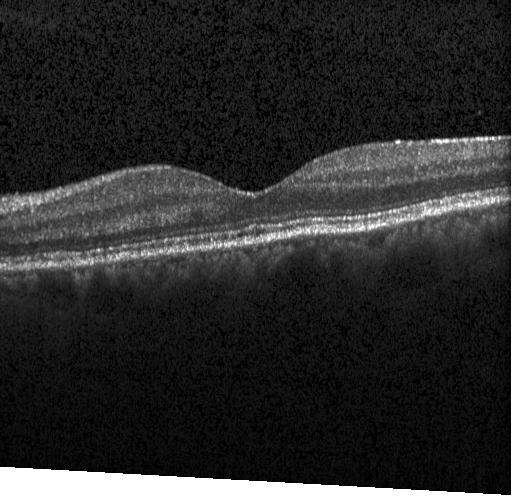 SD-OCT, retinal OCT cross-section. This B-scan demonstrates neither choroidal neovascularization, diabetic macular edema, nor drusen.